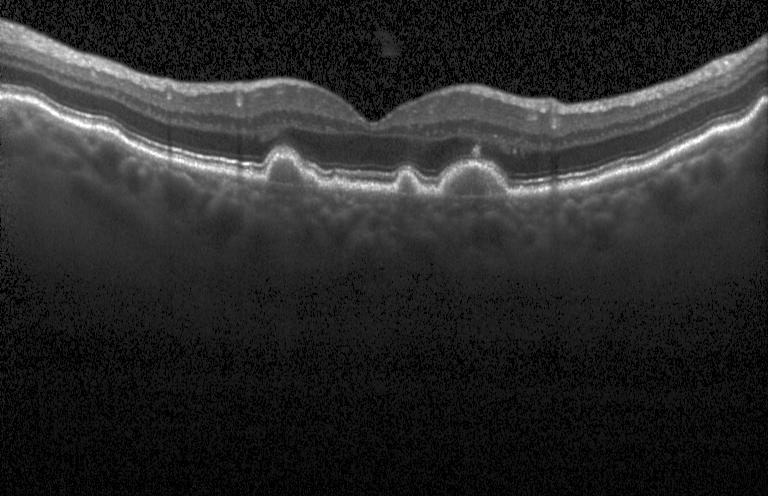
Spectral-domain OCT B-scan: sub-RPE drusenoid deposits.